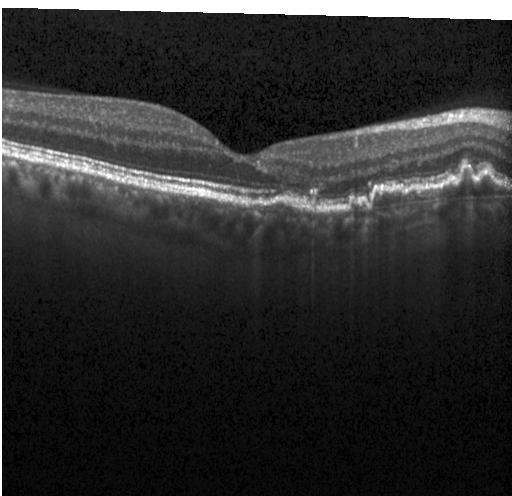 SD-OCT. Fovea-centered. Optical coherence tomography scan. Macular OCT: a choroidal neovascular membrane.